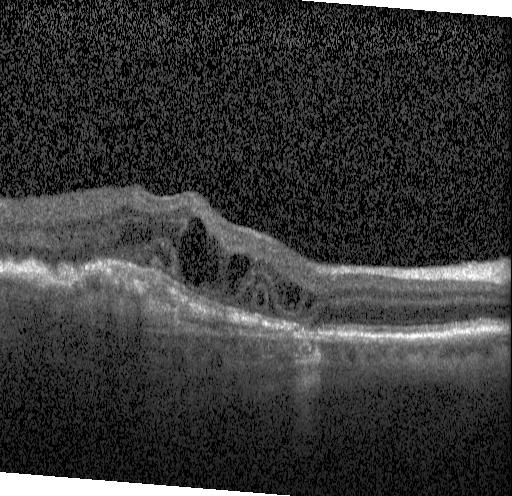
Through the macula; optical coherence tomography B-scan
Impression: a choroidal neovascular membrane.